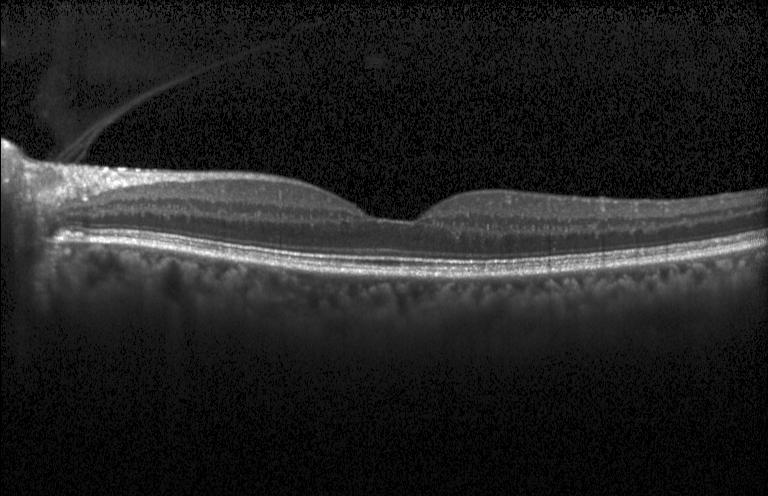 Optical coherence tomography B-scan. SD-OCT. Instrument: Heidelberg Spectralis. Fovea-centered — The scan shows no choroidal neovascularization, diabetic macular edema, or drusen.